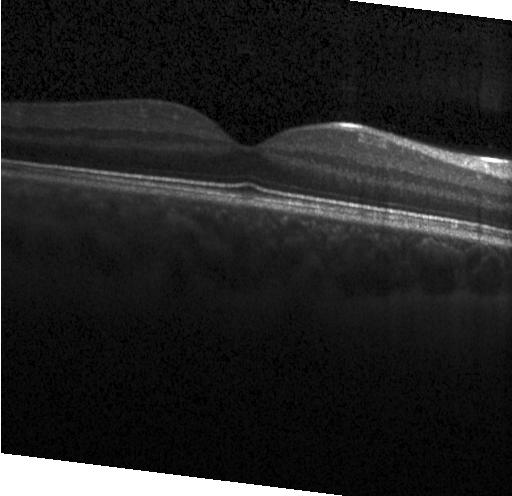 Acquired on a Heidelberg Spectralis · centered on the fovea · spectral-domain OCT · OCT line scan.
The scan shows no evidence of choroidal neovascularization, diabetic macular edema, or drusen.